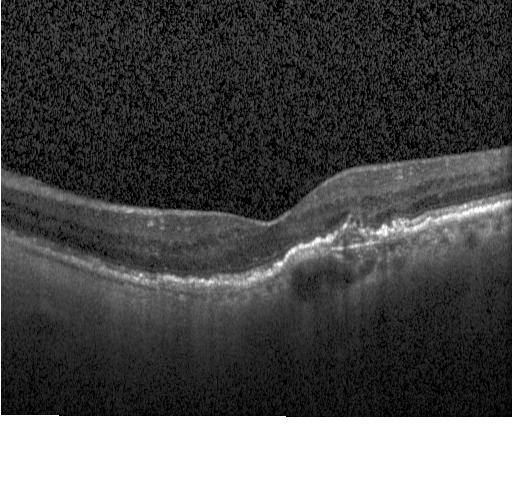
Finding: choroidal neovascularization (CNV).